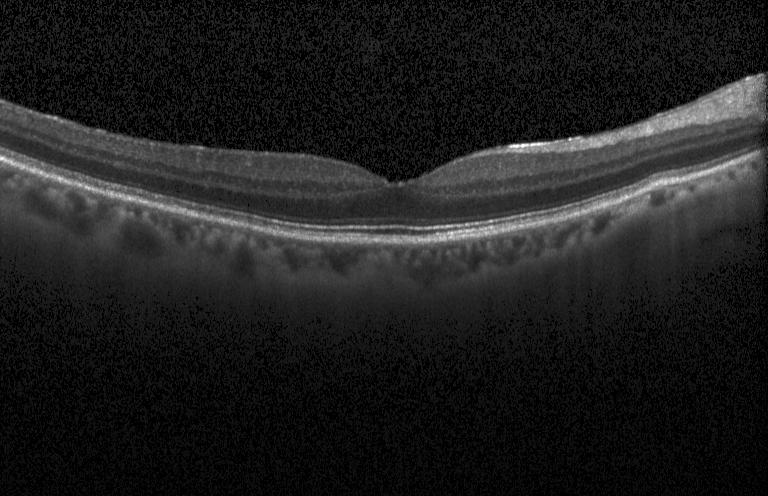

Optical coherence tomography B-scan
No evidence of CNV, DME, or drusen.